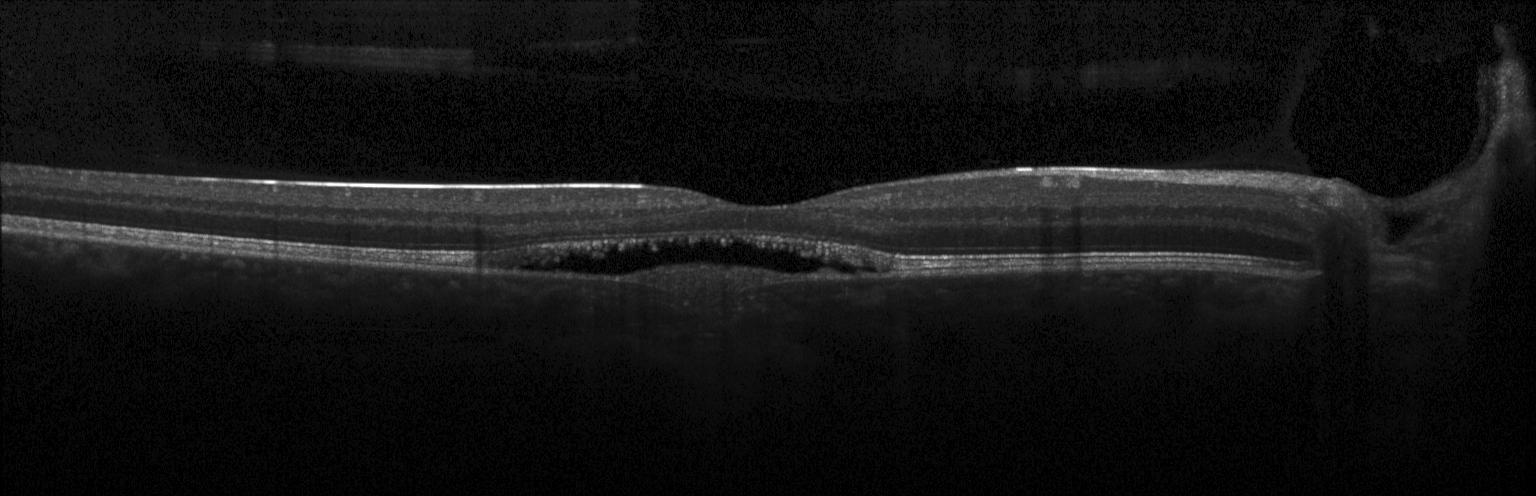
Heidelberg Spectralis OCT system. Spectral-domain optical coherence tomography. Macular scan. OCT B-scan.
Finding: choroidal neovascularization (CNV).